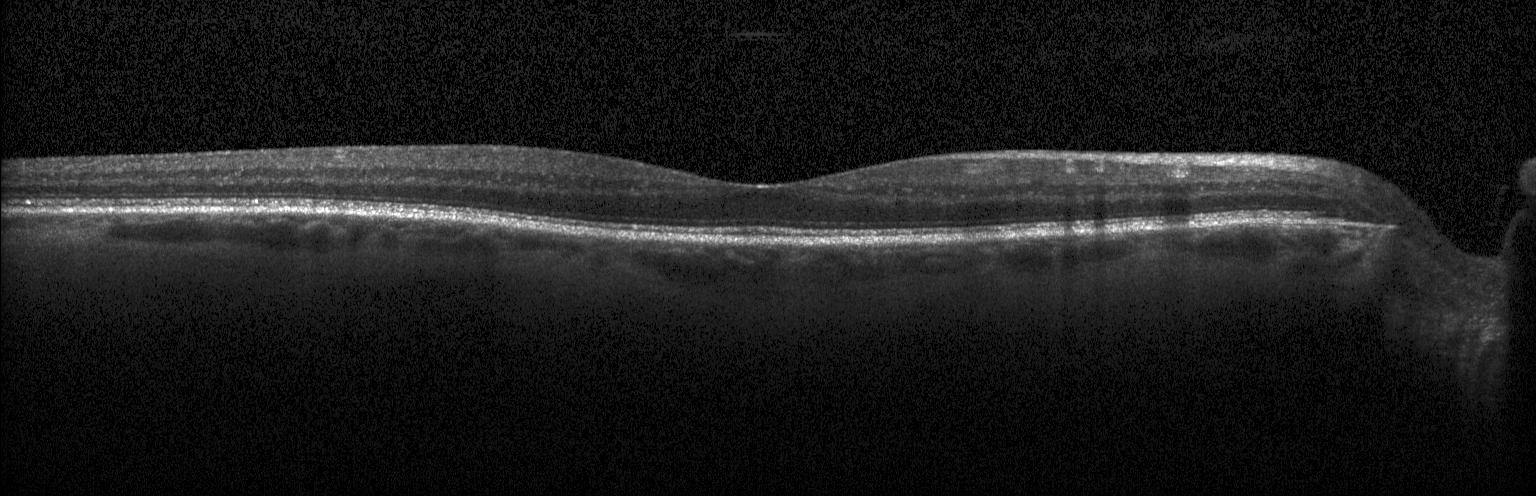

Diagnosis: no evidence of choroidal neovascularization, diabetic macular edema, or drusen.